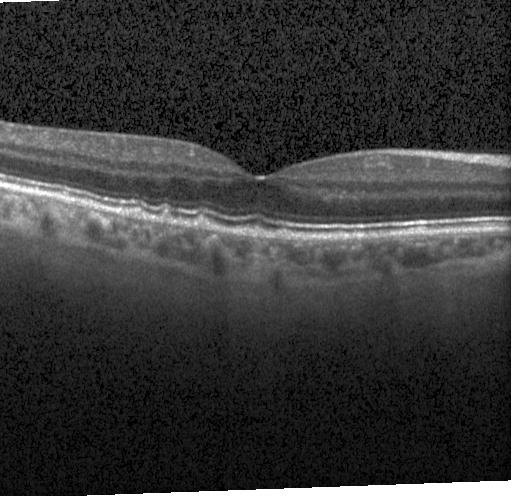 OCT B-scan showing drusen.